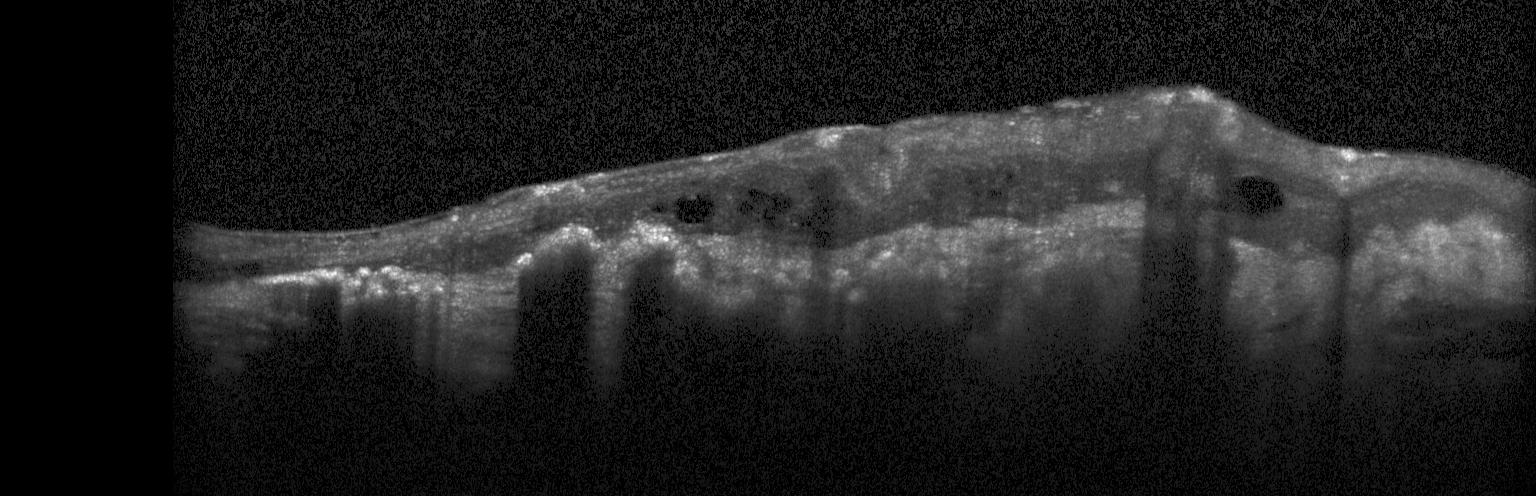 OCT B-scan showing choroidal neovascularization.